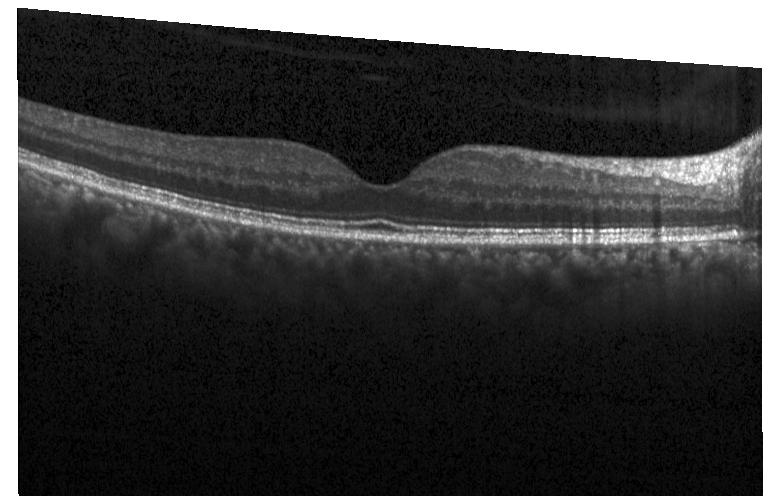
Heidelberg Spectralis OCT system · centered on the fovea · SD-OCT · OCT B-scan.
This B-scan demonstrates neither CNV, DME, nor drusen.